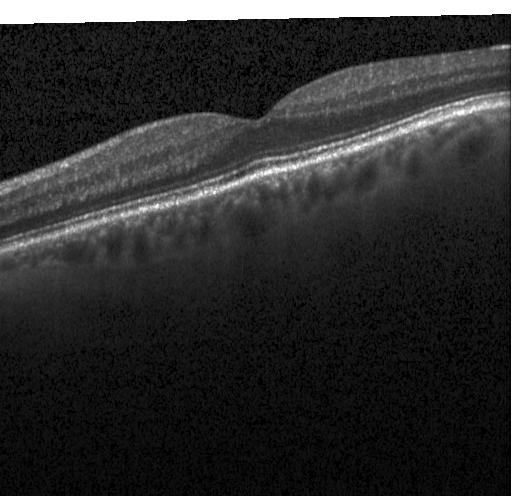
Macular OCT demonstrating no choroidal neovascularization, no diabetic macular edema, and no drusen.